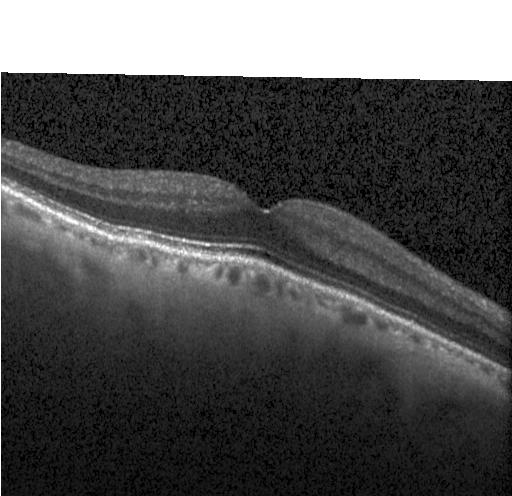

Optical coherence tomography B-scan. This B-scan demonstrates no choroidal neovascularization, no diabetic macular edema, and no drusen.